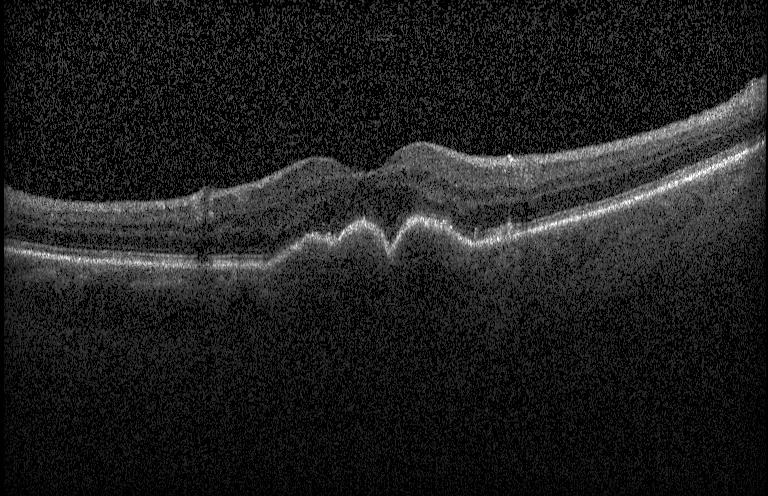
The scan shows choroidal neovascularization (CNV).